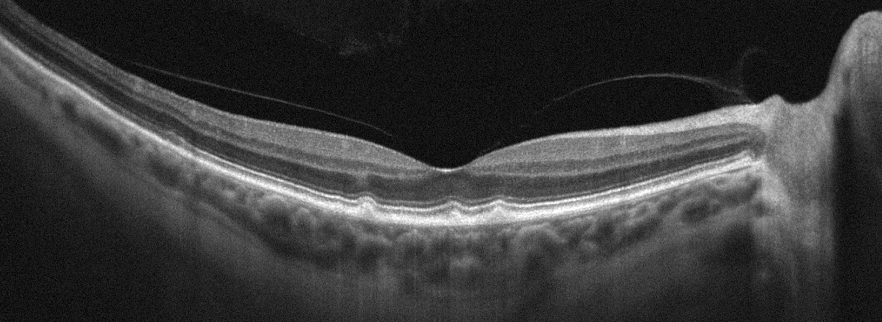 This B-scan demonstrates AMD.